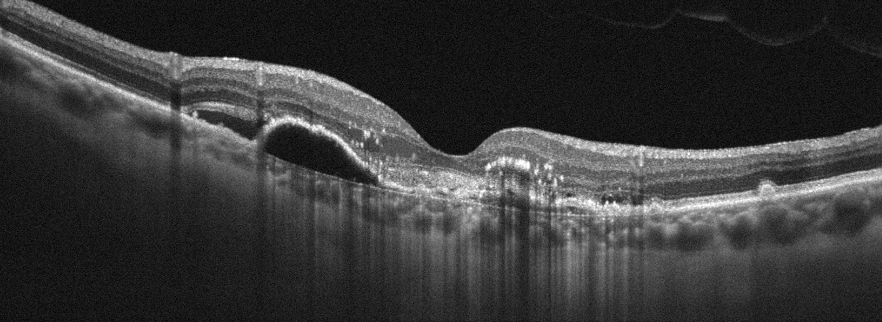

Retinal OCT cross-section, acquired on an Optovue Avanti RTVue XR, oculus dexter
The scan shows age-related macular degeneration (AMD).